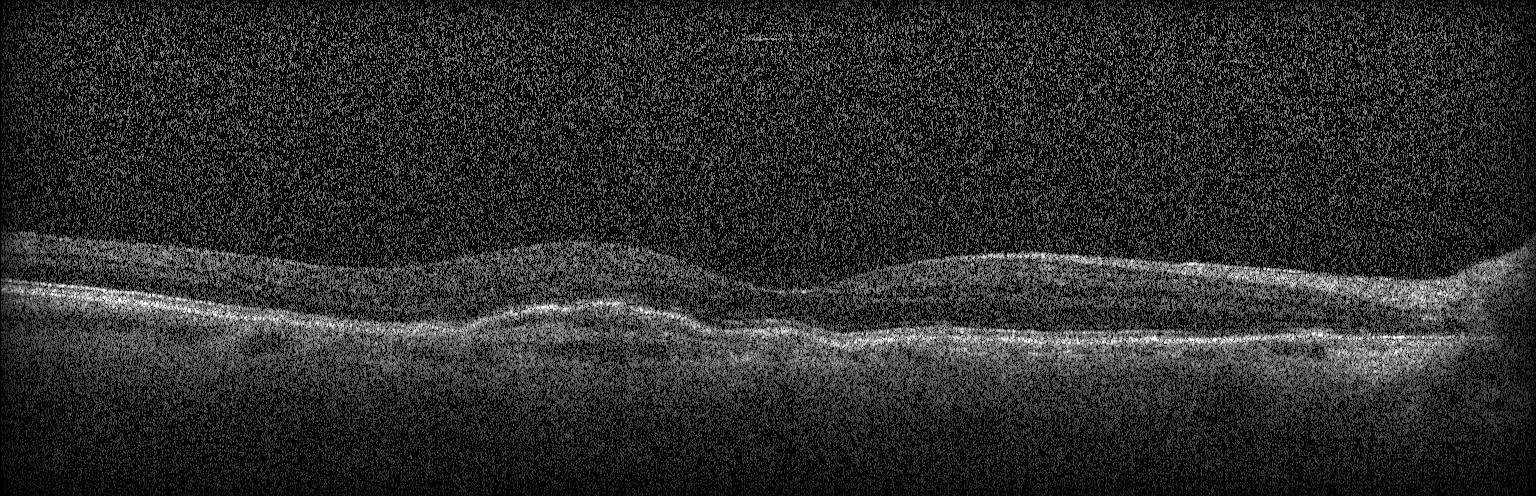
OCT finding: choroidal neovascularization.